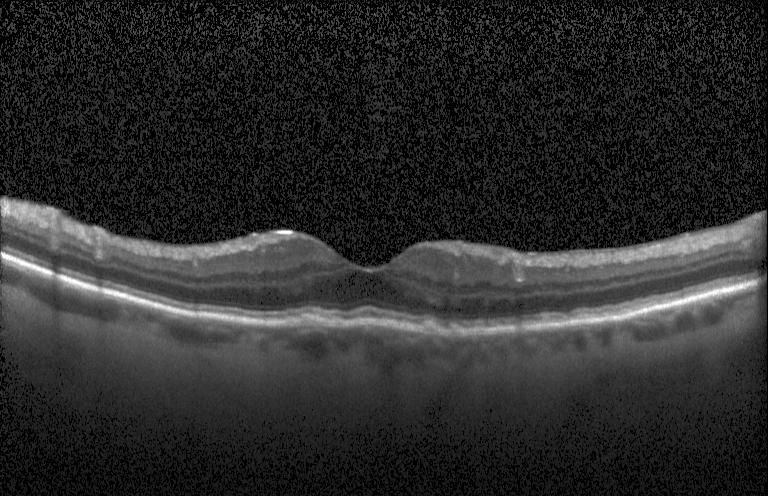

Heidelberg Spectralis; optical coherence tomography scan — Diagnosis: sub-RPE drusenoid deposits.